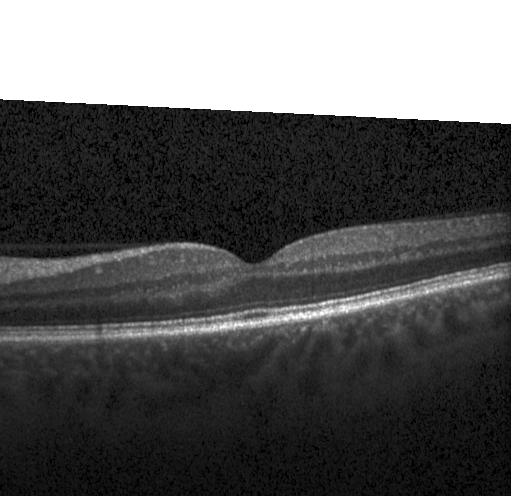
Instrument: Heidelberg Spectralis, SD-OCT, retinal OCT B-scan, fovea-centered — Diagnosis: no evidence of choroidal neovascularization, diabetic macular edema, or drusen.